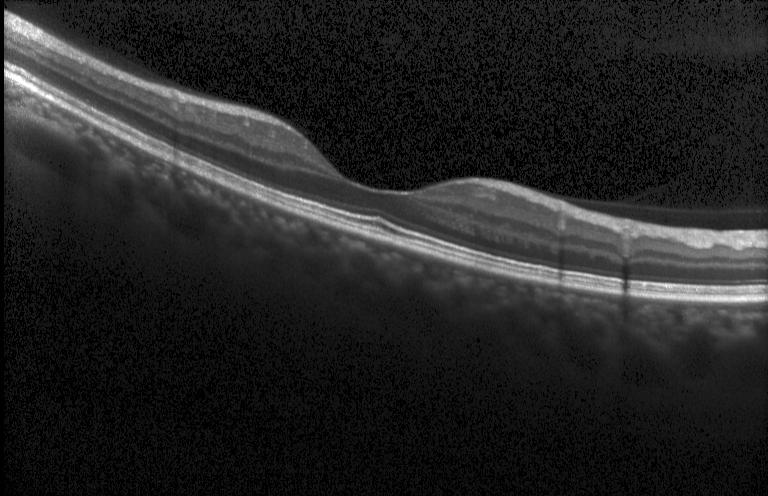

Through the macula. Instrument: Heidelberg Spectralis. Spectral-domain OCT. OCT B-scan. Diagnosis: no CNV, no DME, and no drusen.